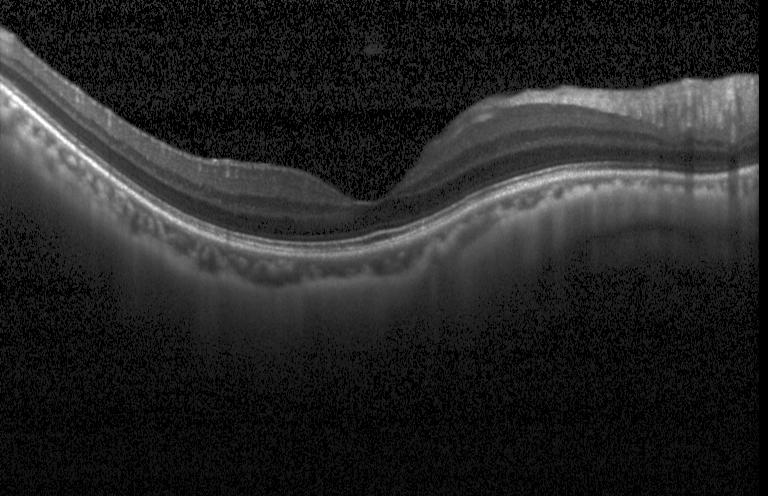 The scan shows no choroidal neovascularization, no diabetic macular edema, and no drusen.